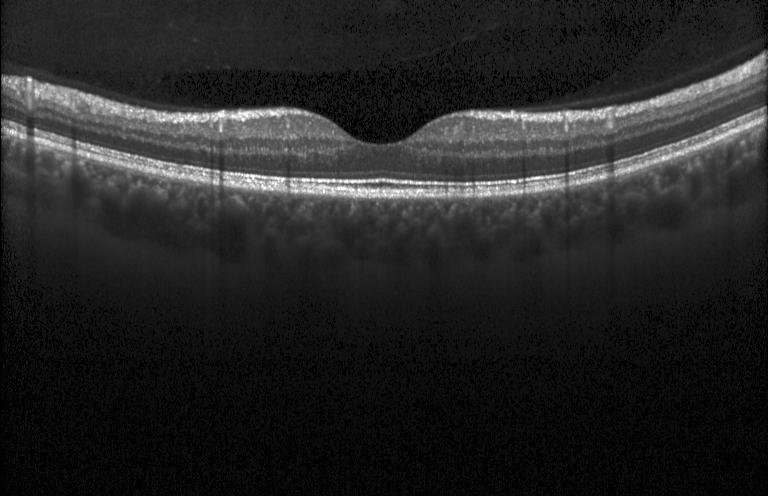
Optical coherence tomography B-scan. Spectral-domain OCT. Centered on the fovea. Heidelberg Spectralis OCT system.
Macular OCT: no evidence of choroidal neovascularization, diabetic macular edema, or drusen.